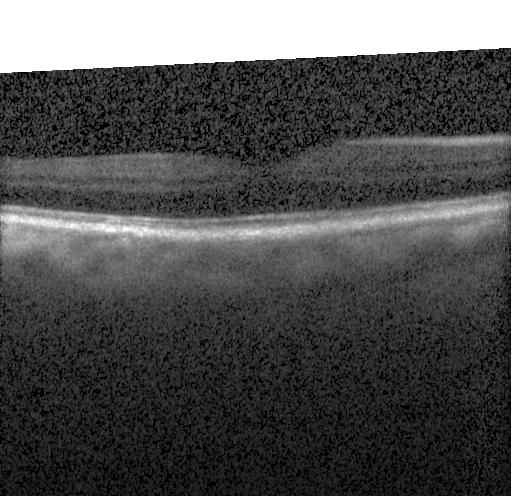

Centered on the fovea, Heidelberg Spectralis OCT system, optical coherence tomography B-scan, SD-OCT. Assessment: no evidence of CNV, DME, or drusen.